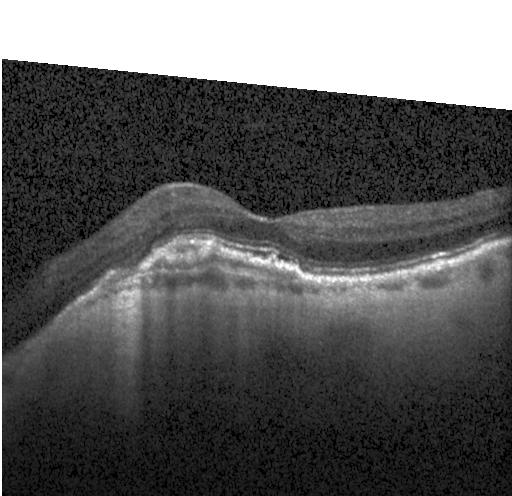 Macular OCT: a choroidal neovascular membrane.